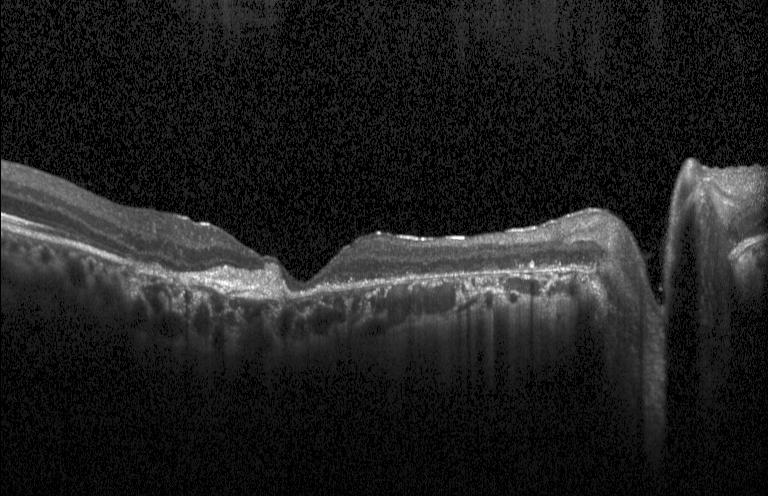
Optical coherence tomography B-scan. Macular scan — Dx: a choroidal neovascular membrane.